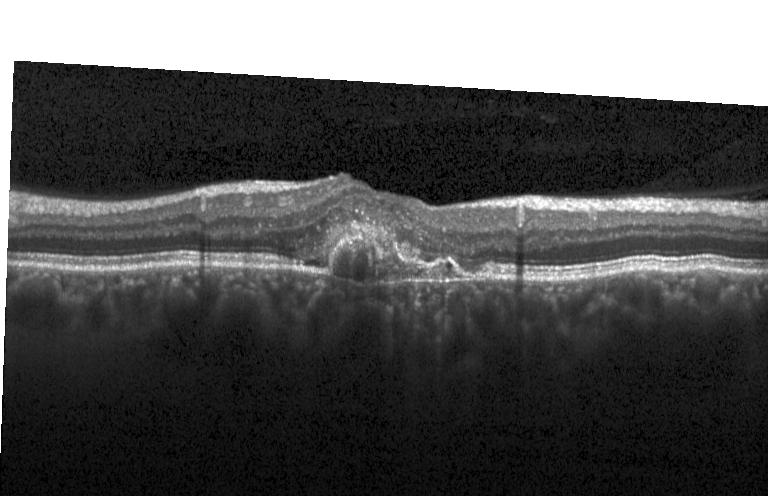
Acquired on a Heidelberg Spectralis. SD-OCT. Optical coherence tomography scan. Finding: CNV.